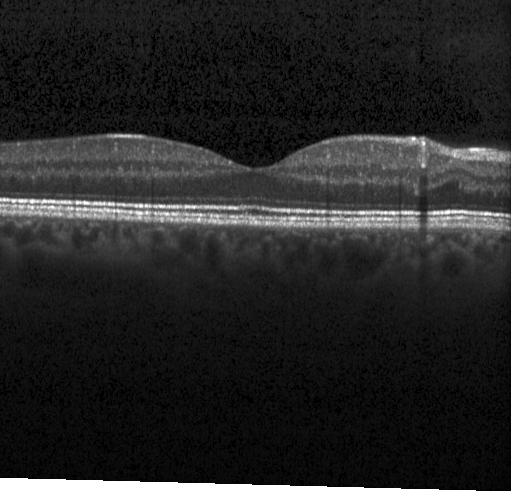 Impression: no CNV, DME, or drusen.